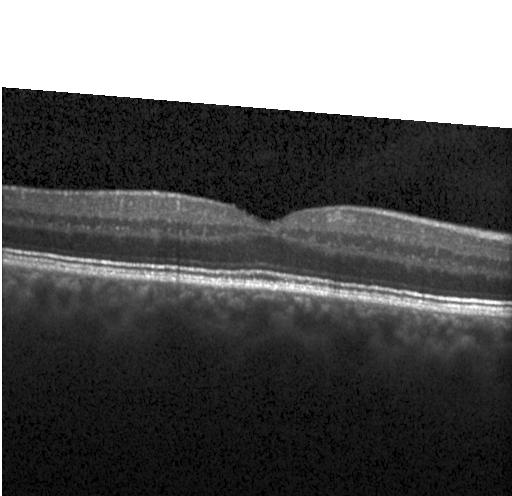 Assessment: no choroidal neovascularization, no diabetic macular edema, and no drusen.